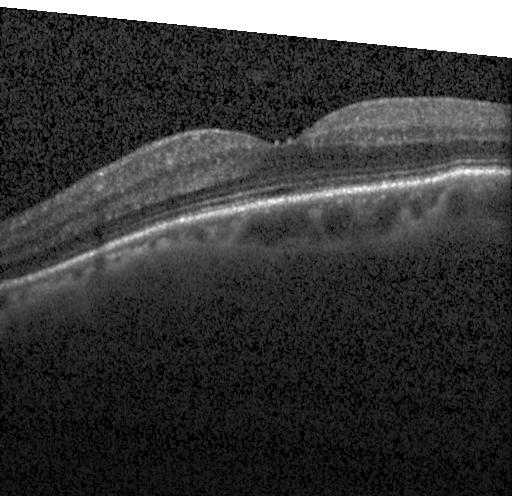
OCT finding: no evidence of choroidal neovascularization, diabetic macular edema, or drusen.